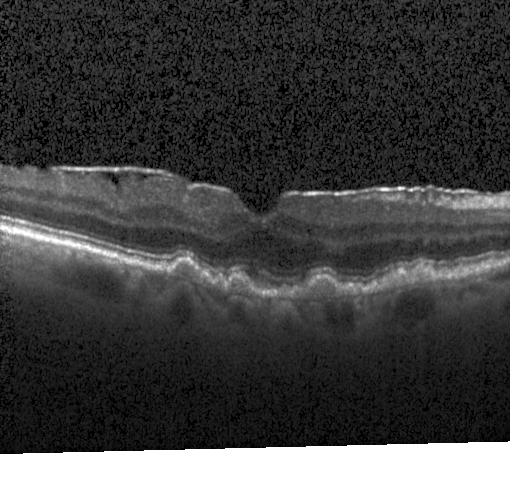
Heidelberg Spectralis, OCT B-scan. Assessment: drusen.